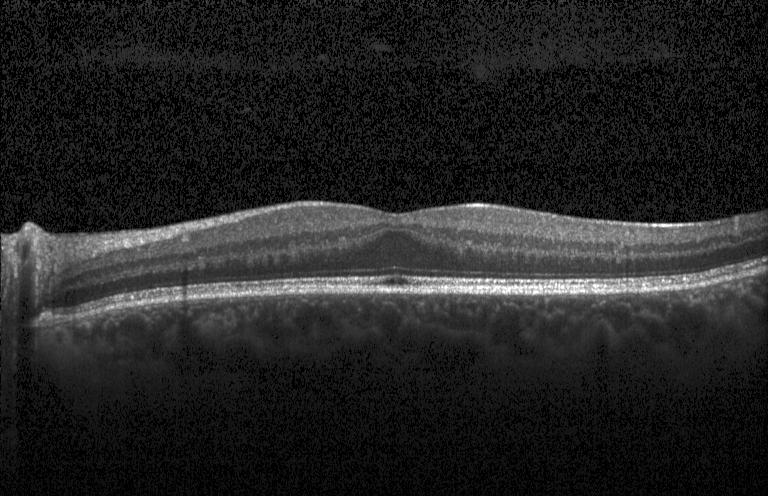

Macular OCT: no evidence of choroidal neovascularization, diabetic macular edema, or drusen.